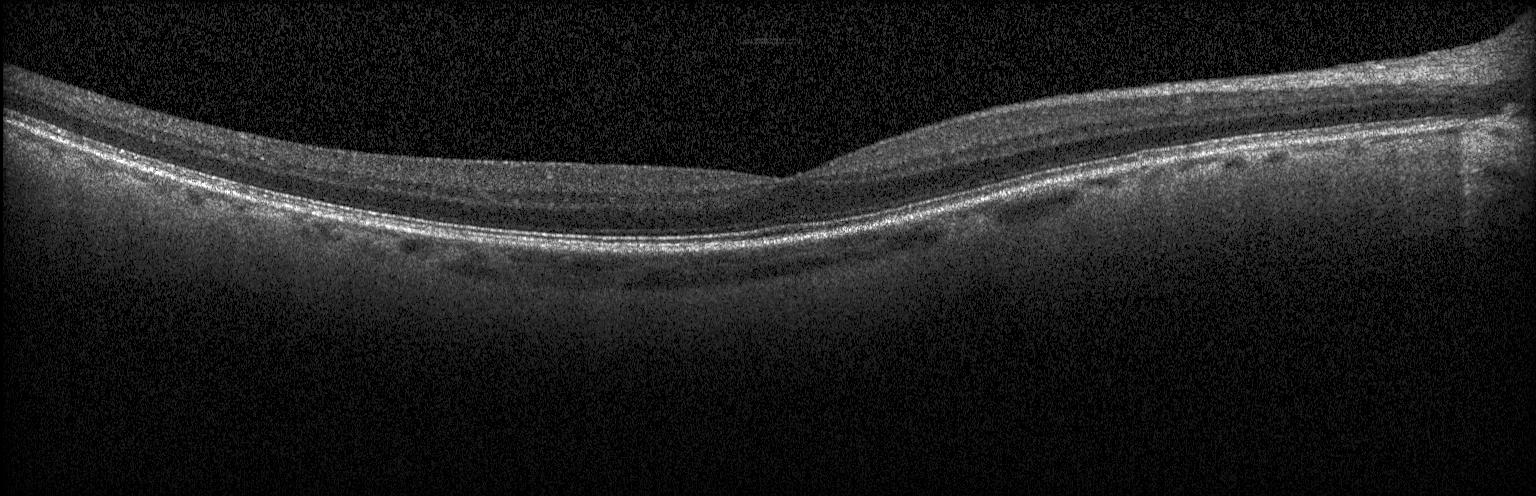

Impression: no choroidal neovascularization, no diabetic macular edema, and no drusen.